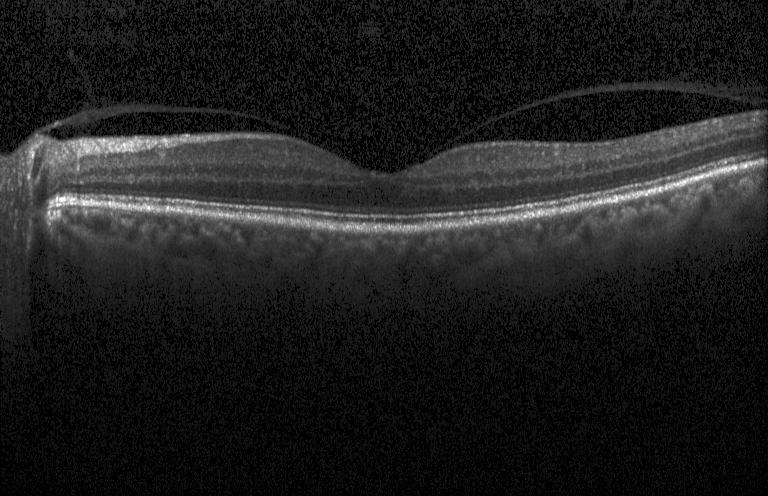

Centered on the fovea. Optical coherence tomography B-scan. This B-scan demonstrates neither CNV, DME, nor drusen.